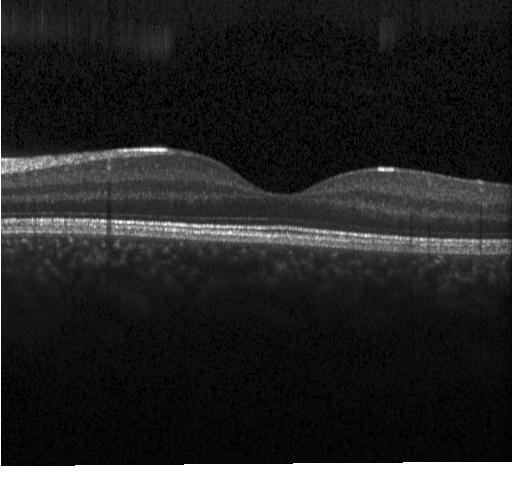

Retinal OCT cross-section, spectral-domain OCT, fovea-centered.
Neither CNV, DME, nor drusen.